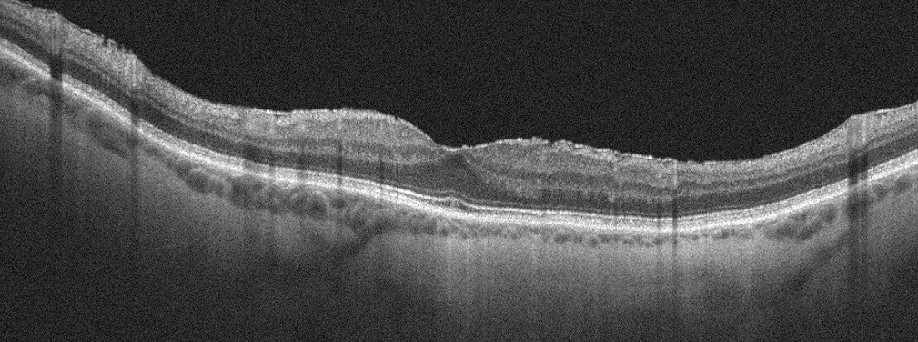 OCT B-scan showing ERM.